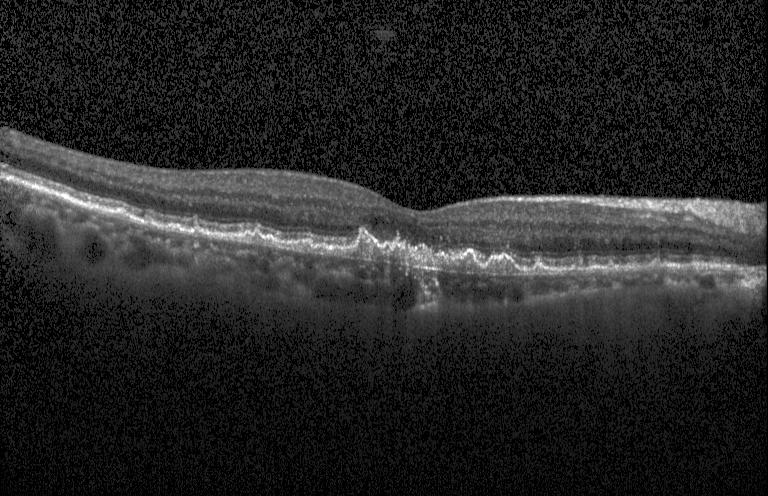
OCT scan showing a choroidal neovascular membrane.